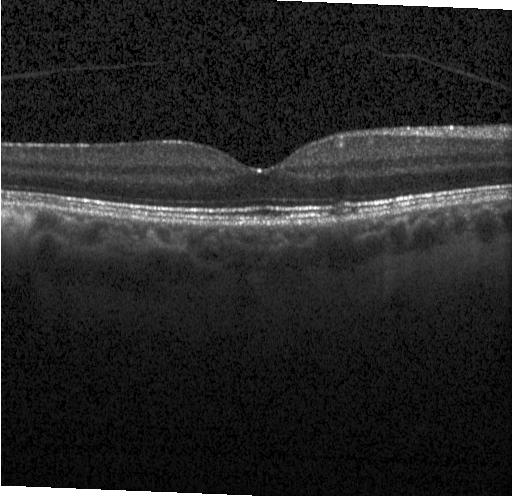
Centered on the fovea. Retinal OCT B-scan. Spectral-domain optical coherence tomography
Sub-RPE drusenoid deposits.